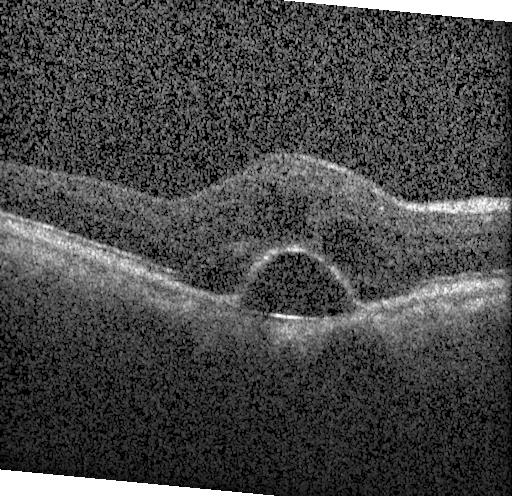

Retinal OCT cross-section. Heidelberg Spectralis OCT system.
Finding: choroidal neovascularization (CNV).